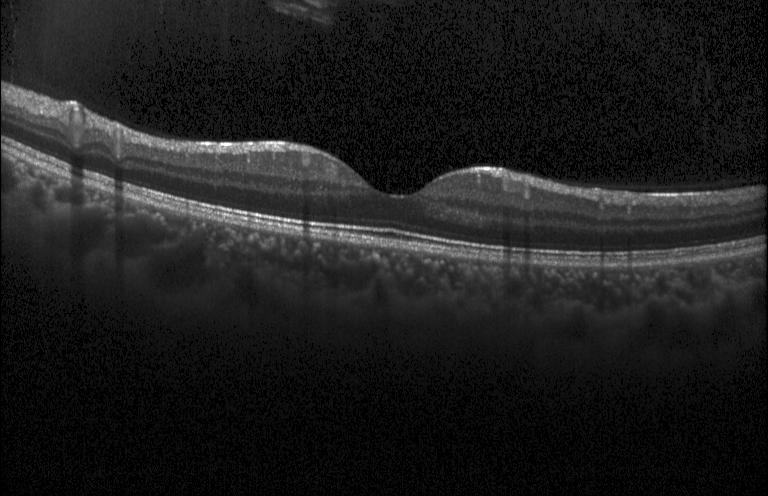 Dx: no CNV, no DME, and no drusen.